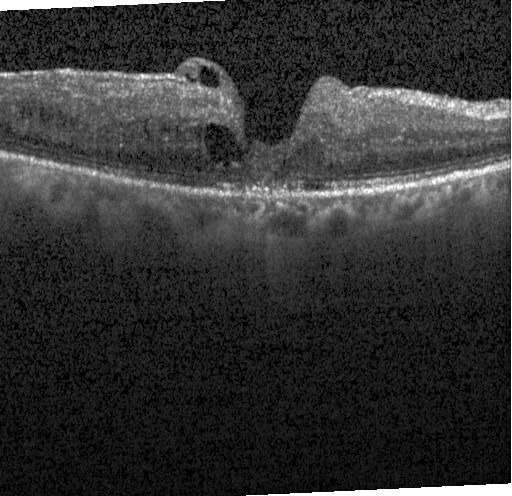

Assessment: diabetic macular edema (DME).